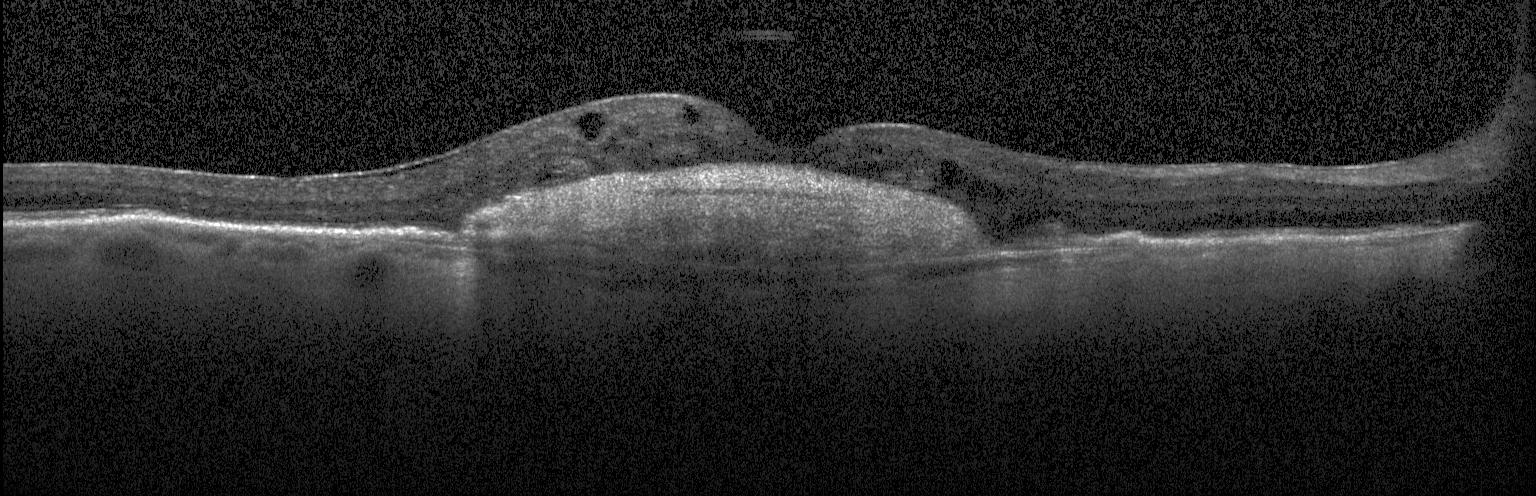
Assessment: CNV.